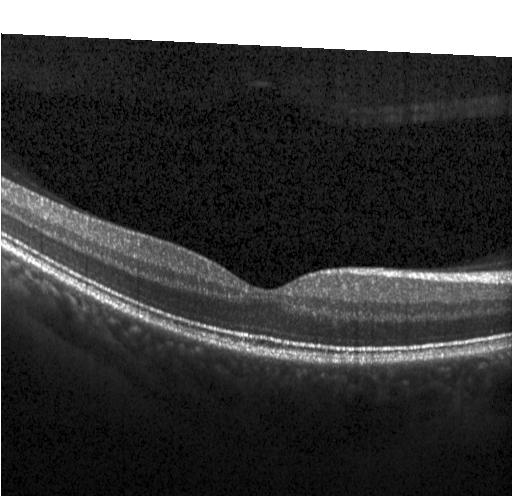
Impression: no choroidal neovascularization, diabetic macular edema, or drusen.